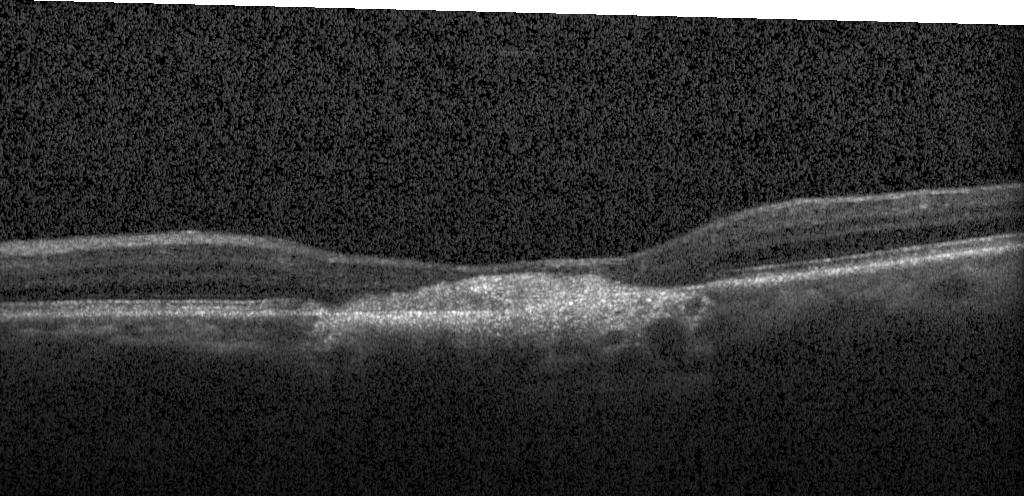
Optical coherence tomography B-scan
Dx: choroidal neovascularization (CNV).